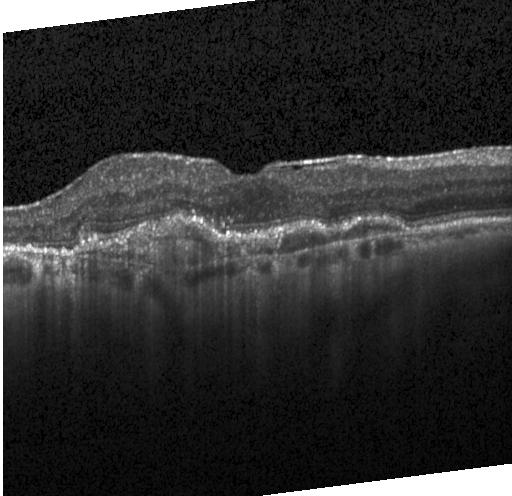
Diagnosis: a choroidal neovascular membrane.